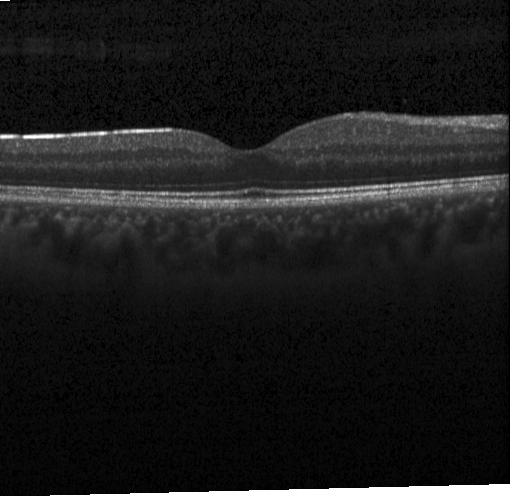
Instrument: Heidelberg Spectralis, spectral-domain optical coherence tomography, optical coherence tomography B-scan, through the macula.
No choroidal neovascularization, diabetic macular edema, or drusen.